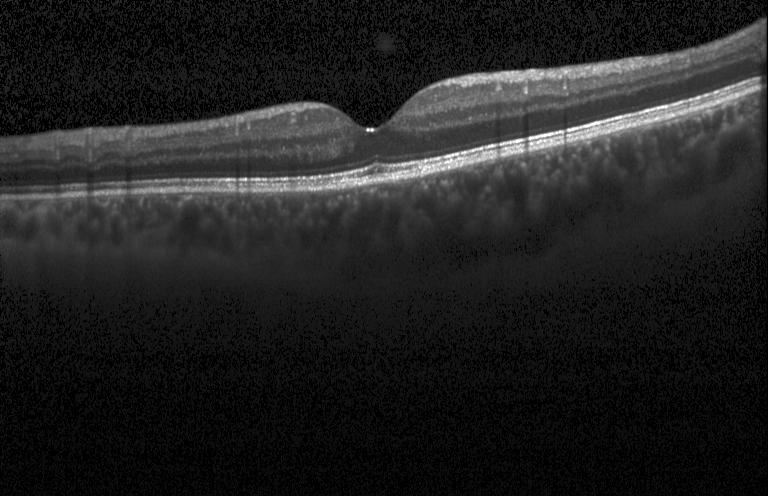
OCT line scan. Centered on the fovea. Heidelberg Spectralis OCT system — OCT finding: neither choroidal neovascularization, diabetic macular edema, nor drusen.